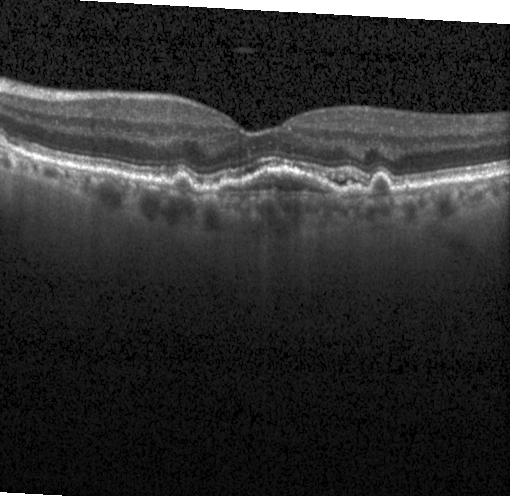

Heidelberg Spectralis OCT system, optical coherence tomography B-scan, through the macula. Impression: a choroidal neovascular membrane.